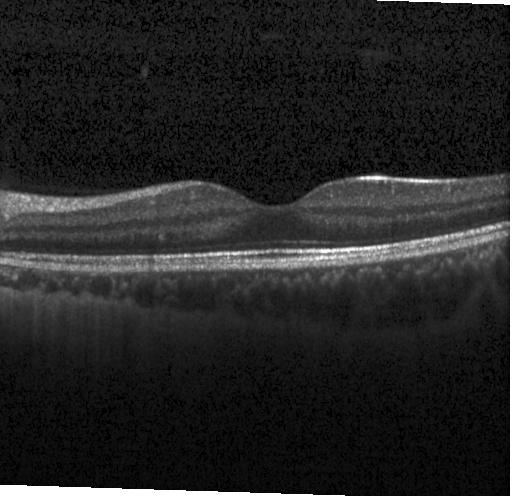 Heidelberg Spectralis, retinal OCT cross-section. Dx: no CNV, DME, or drusen.